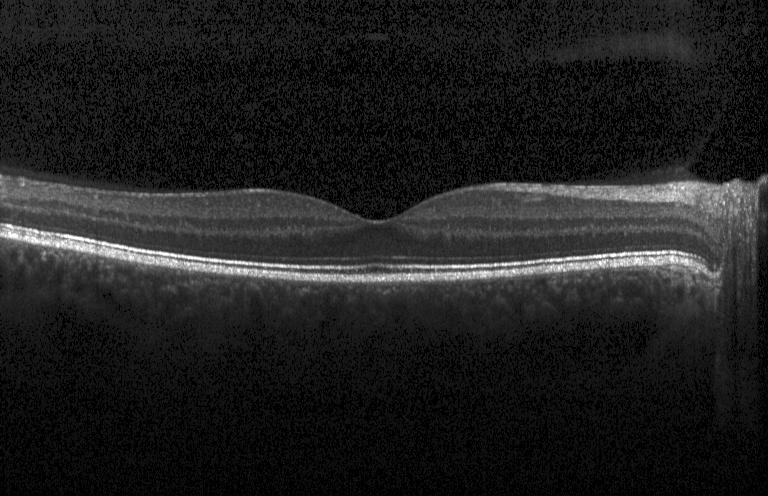 SD-OCT. Fovea-centered. OCT B-scan. Acquired on a Heidelberg Spectralis
Diagnosis: neither choroidal neovascularization, diabetic macular edema, nor drusen.